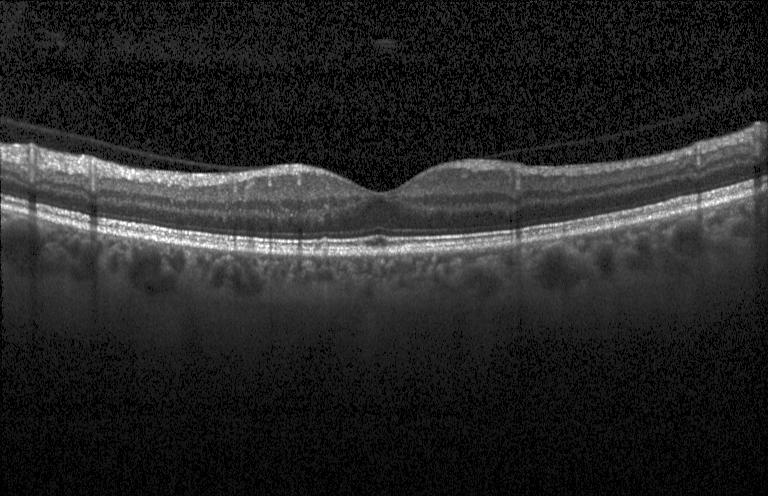
Diagnosis: no evidence of choroidal neovascularization, diabetic macular edema, or drusen.